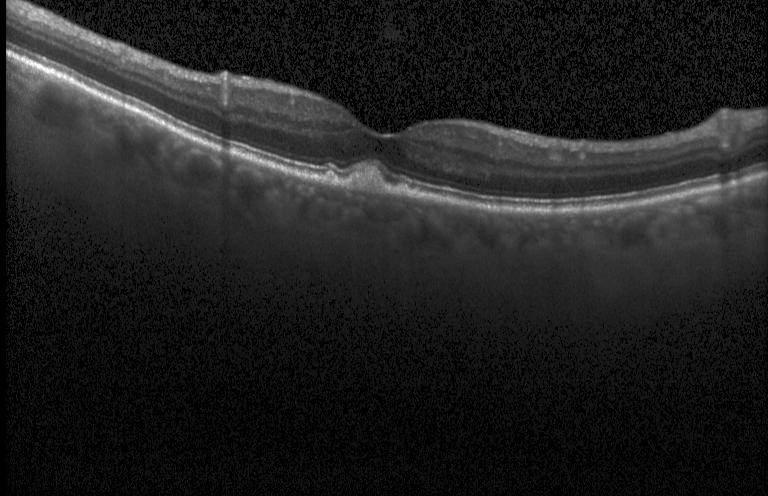 Retinal OCT cross-section · horizontal scan through the fovea · spectral-domain OCT.
OCT finding: multiple drusen.